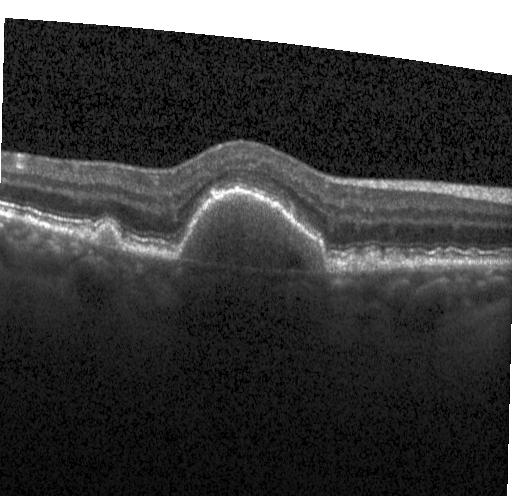
Macular scan. OCT line scan. A choroidal neovascular membrane.